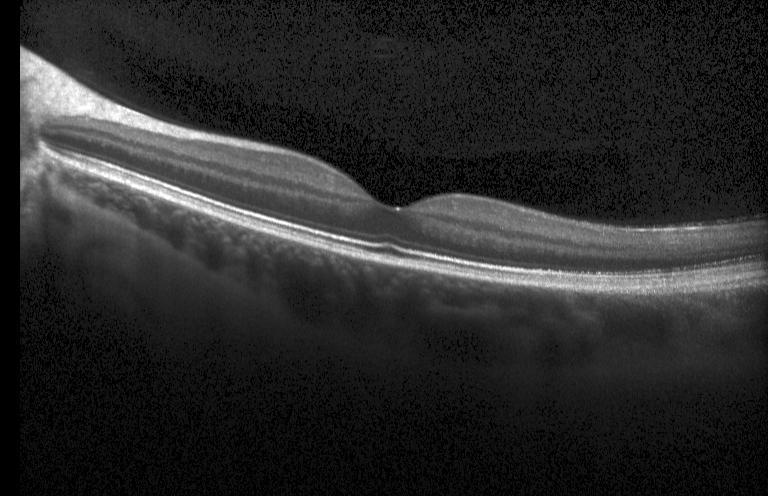

Assessment: no evidence of CNV, DME, or drusen.